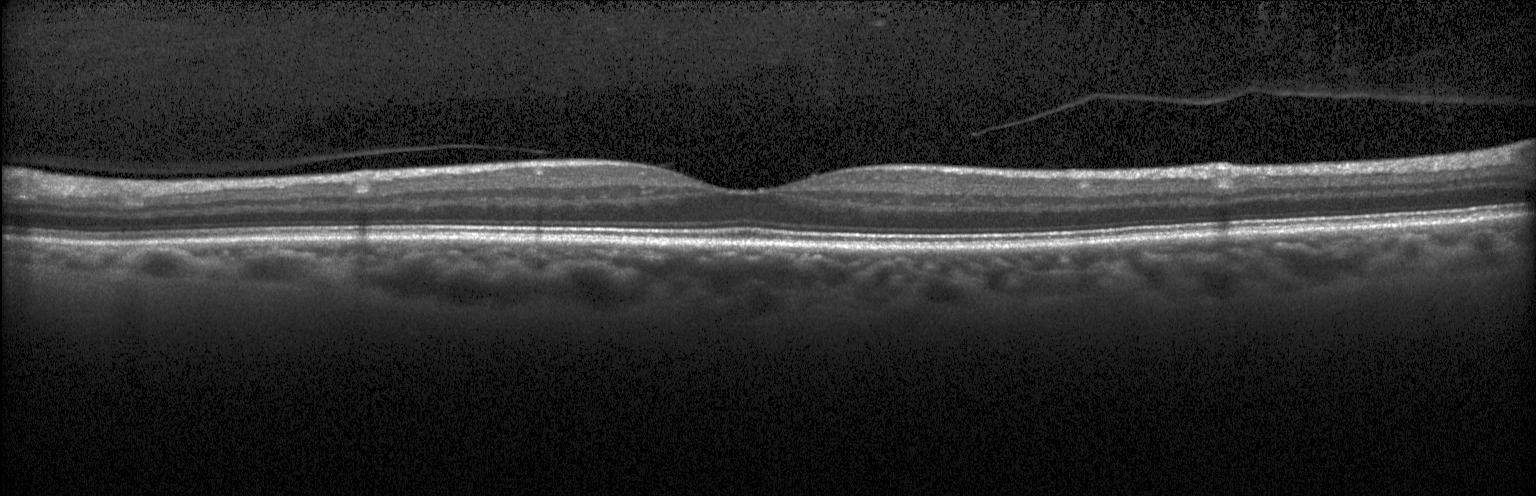 Impression: neither choroidal neovascularization, diabetic macular edema, nor drusen.